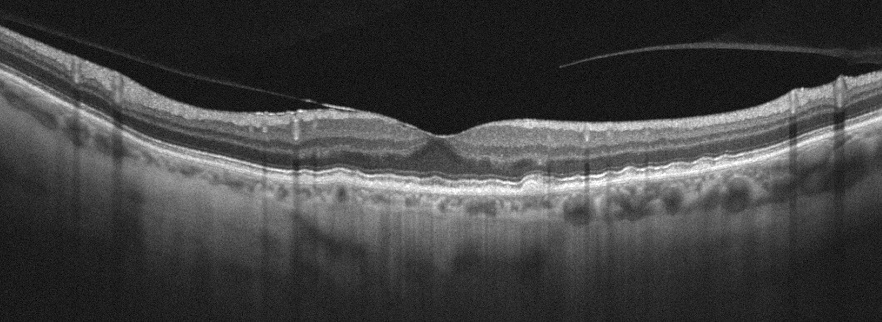

Finding: AMD.